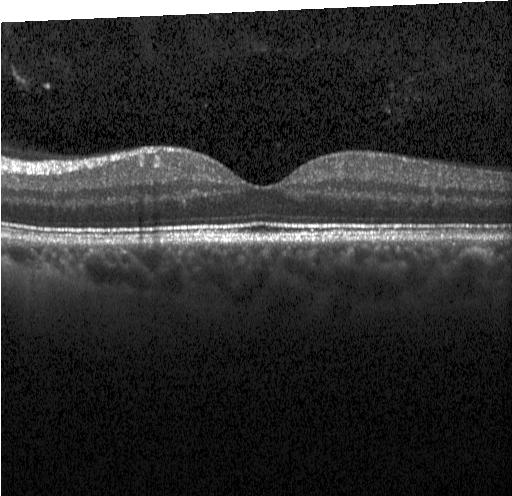

Retinal OCT B-scan — Impression: no evidence of choroidal neovascularization, diabetic macular edema, or drusen.